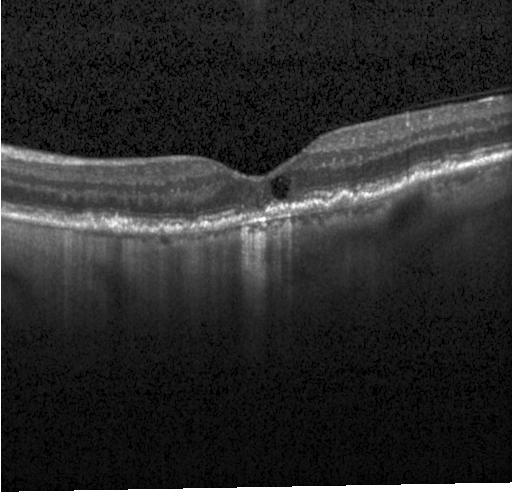

Centered on the fovea. Instrument: Heidelberg Spectralis. SD-OCT. OCT line scan — This B-scan demonstrates a choroidal neovascular membrane.